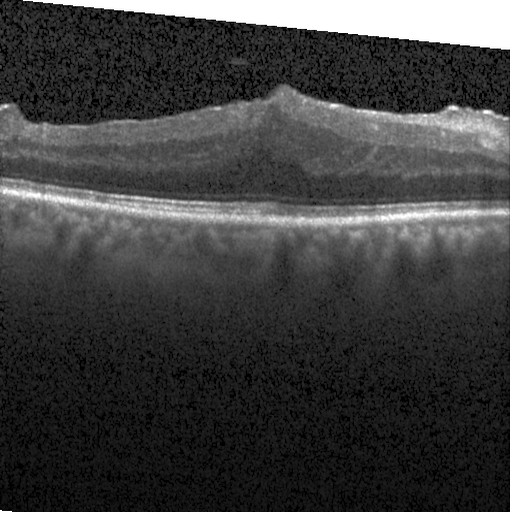

Spectral-domain optical coherence tomography; through the macula; retinal OCT B-scan; Heidelberg Spectralis OCT system
Finding: diabetic macular edema.